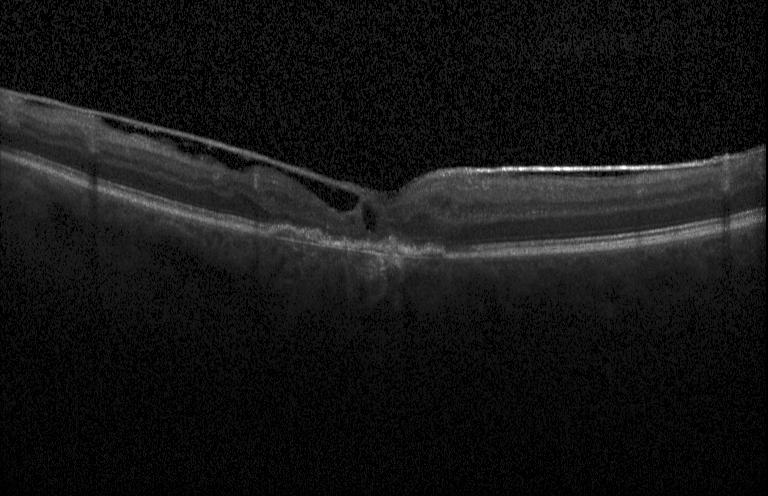

SD-OCT; centered on the fovea; OCT B-scan.
OCT finding: CNV.